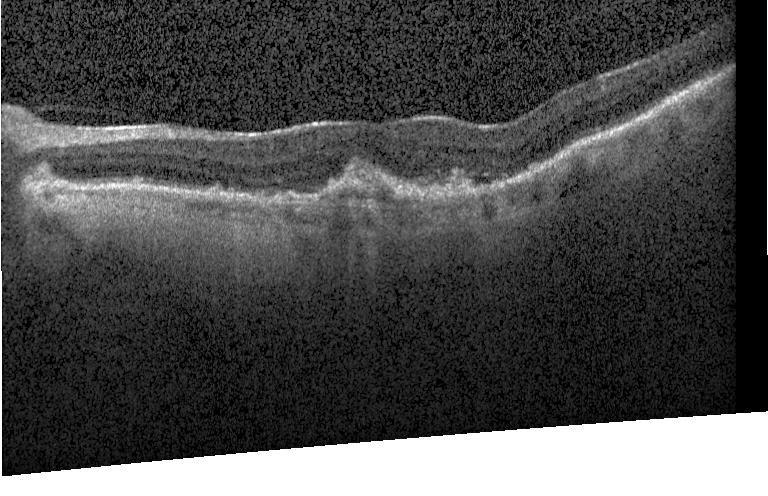

Optical coherence tomography scan, Heidelberg Spectralis OCT system, spectral-domain optical coherence tomography
Finding: a choroidal neovascular membrane.